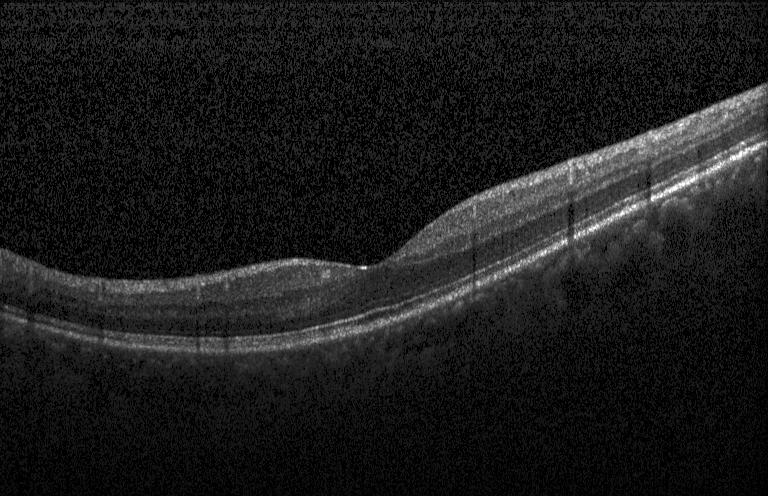
OCT line scan, spectral-domain optical coherence tomography, acquired on a Heidelberg Spectralis, through the macula — OCT finding: neither CNV, DME, nor drusen.